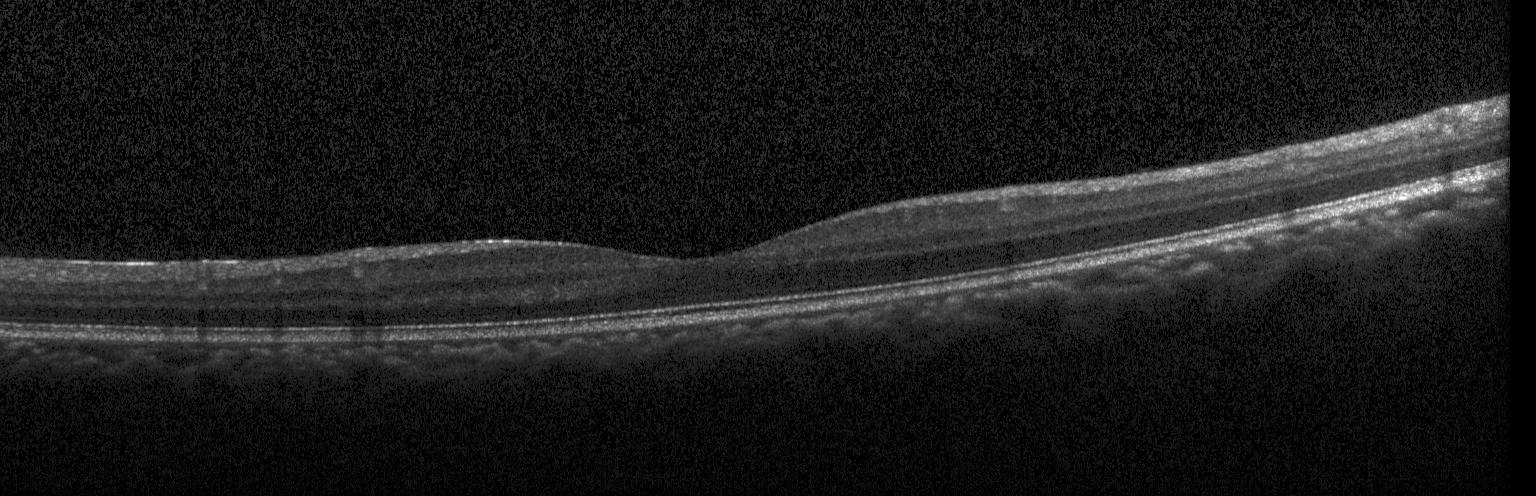

Retinal OCT B-scan
Dx: no evidence of choroidal neovascularization, diabetic macular edema, or drusen.